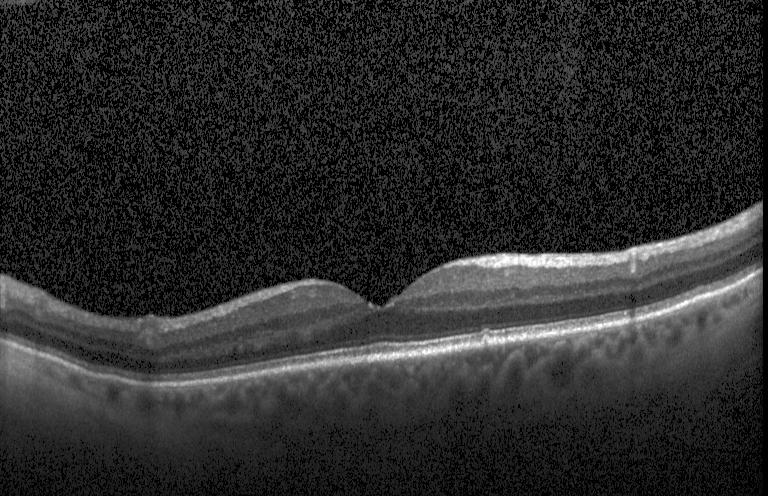
Horizontal scan through the fovea. Retinal OCT cross-section. Instrument: Heidelberg Spectralis — Diagnosis: sub-RPE drusenoid deposits.